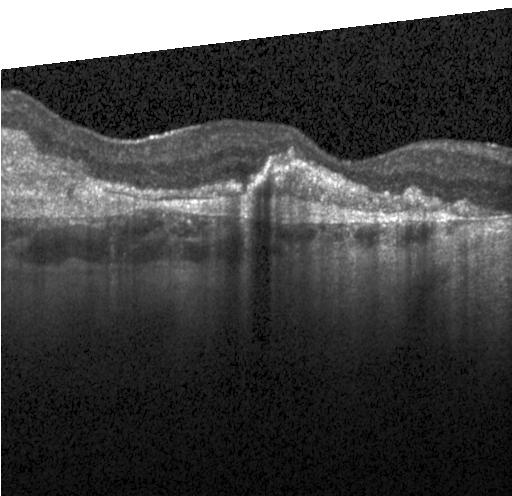
Spectral-domain OCT B-scan: choroidal neovascularization (CNV).